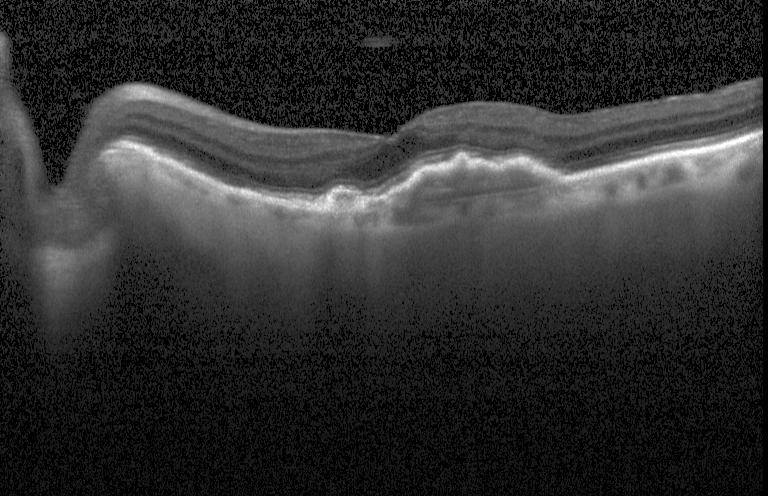 Optical coherence tomography scan. Diagnosis: a choroidal neovascular membrane.